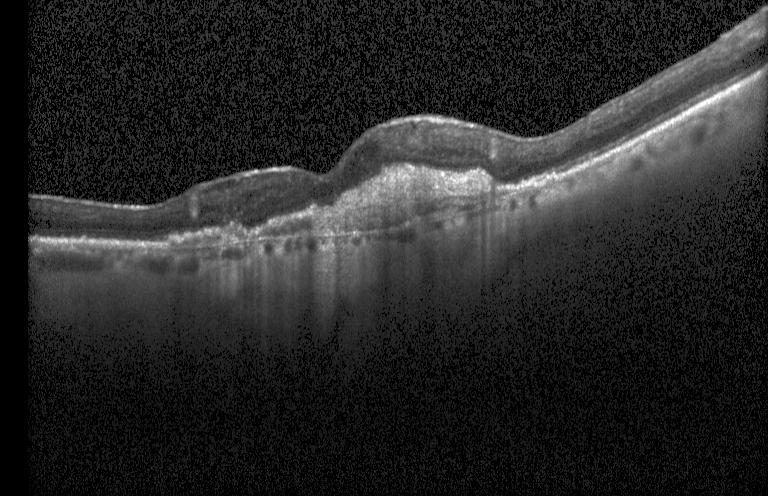

Spectral-domain optical coherence tomography; instrument: Heidelberg Spectralis; optical coherence tomography B-scan. Diagnosis: choroidal neovascularization.